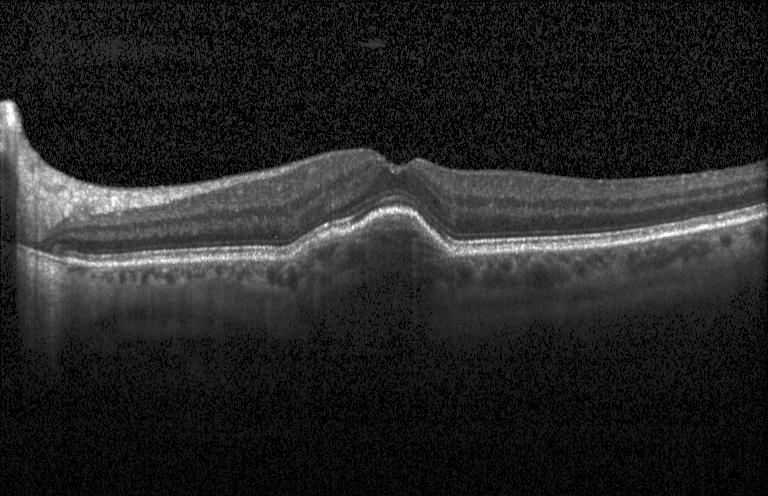

OCT finding: a choroidal neovascular membrane.